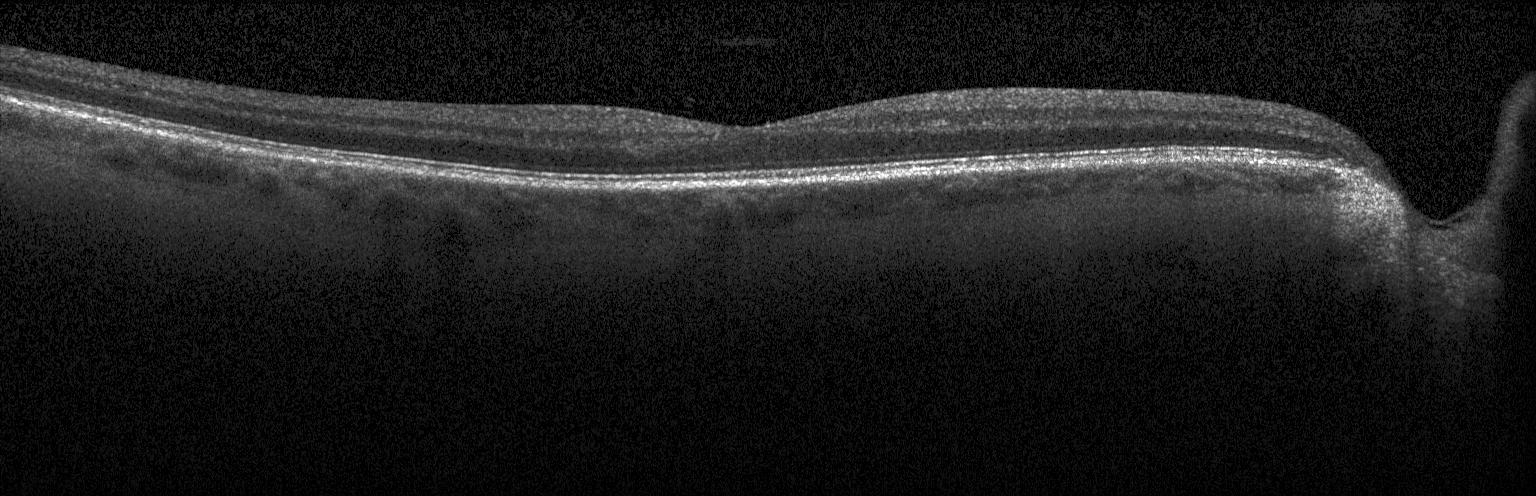

OCT line scan. Through the macula — Dx: neither choroidal neovascularization, diabetic macular edema, nor drusen.